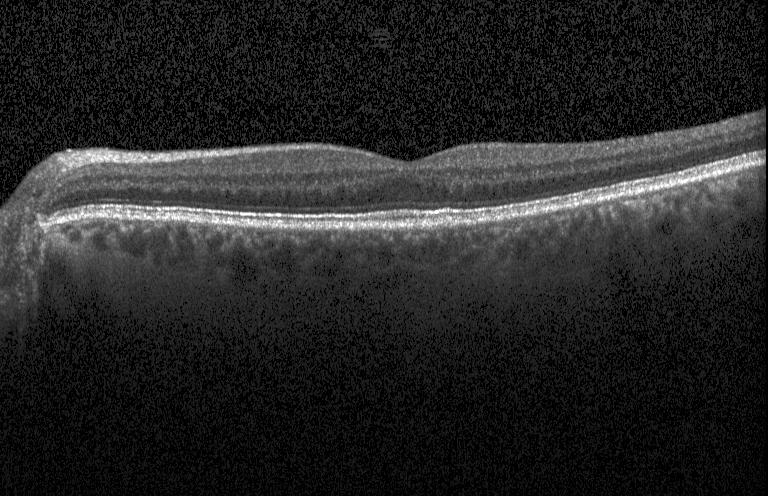

Instrument: Heidelberg Spectralis; macular scan; spectral-domain optical coherence tomography; retinal OCT B-scan. Assessment: no evidence of CNV, DME, or drusen.